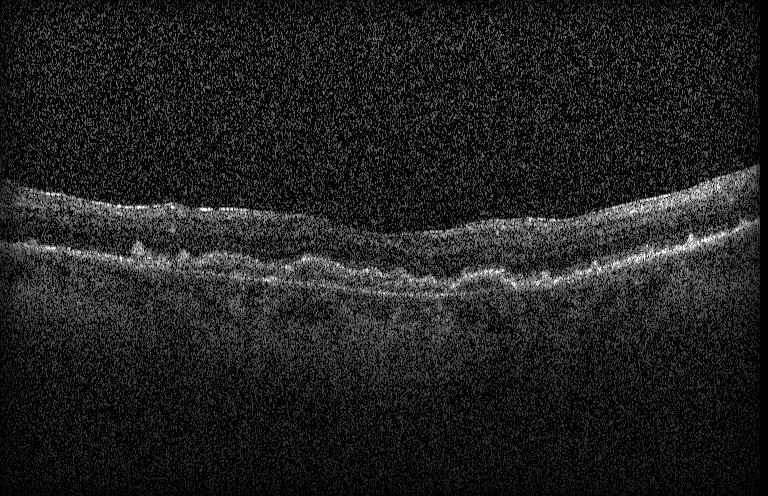
Optical coherence tomography B-scan — Diagnosis: a choroidal neovascular membrane.